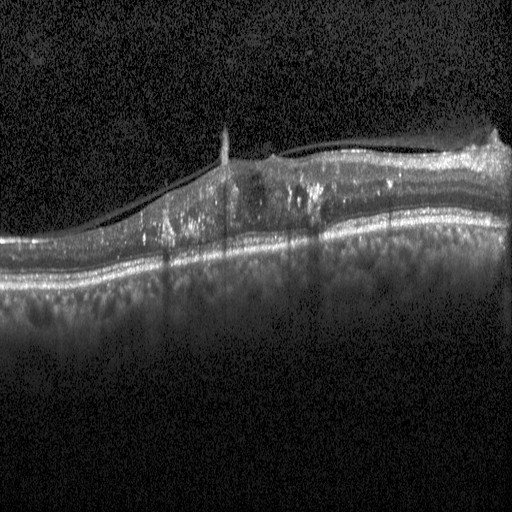
Retinal OCT cross-section showing diabetic macular edema.